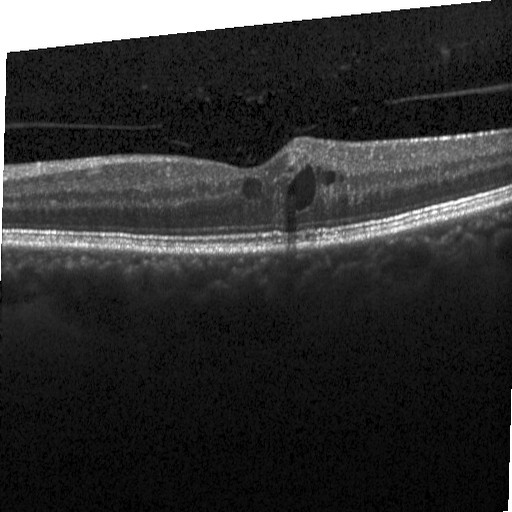
Macular OCT: DME.